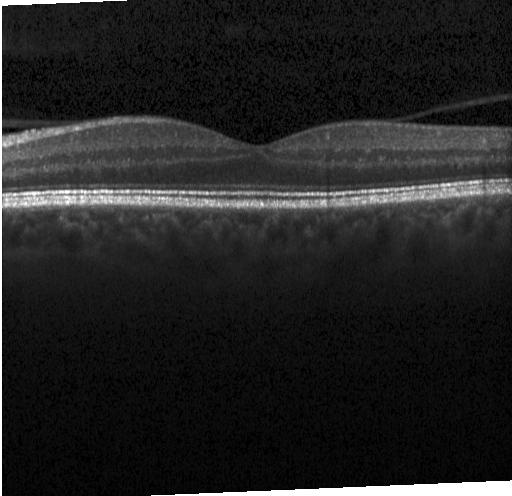 Optical coherence tomography B-scan · spectral-domain OCT.
This B-scan demonstrates no evidence of choroidal neovascularization, diabetic macular edema, or drusen.